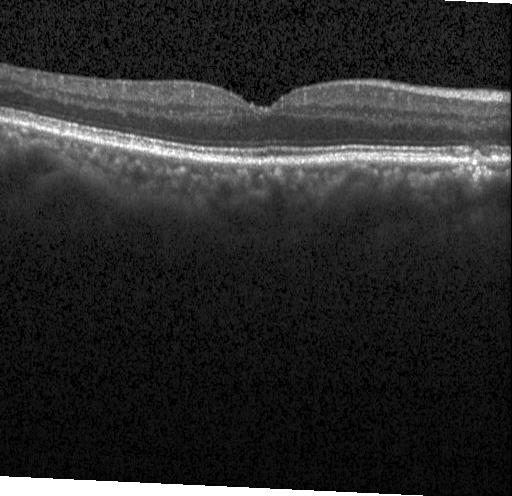
Fovea-centered, retinal OCT B-scan, Heidelberg Spectralis OCT system, spectral-domain OCT.
Impression: no evidence of choroidal neovascularization, diabetic macular edema, or drusen.